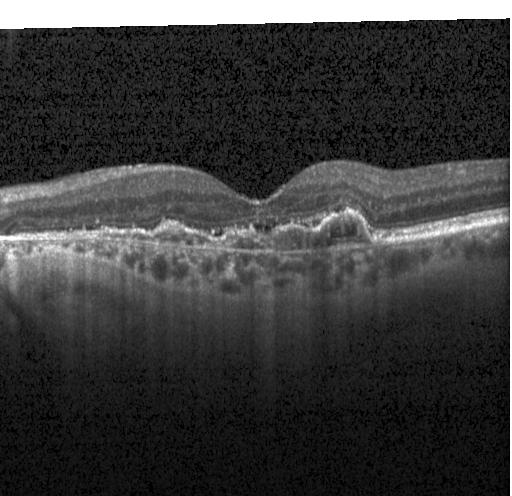

A choroidal neovascular membrane.